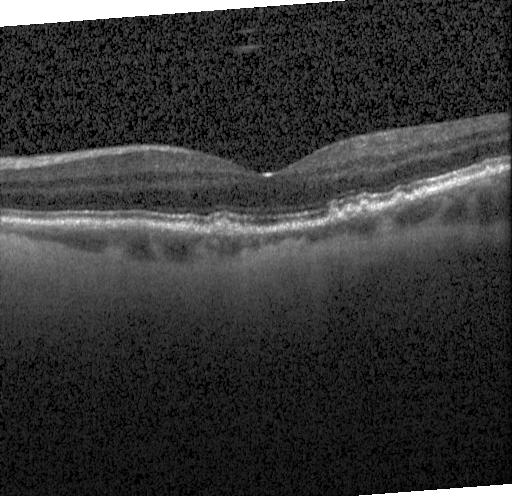
Optical coherence tomography scan
Impression: drusen.